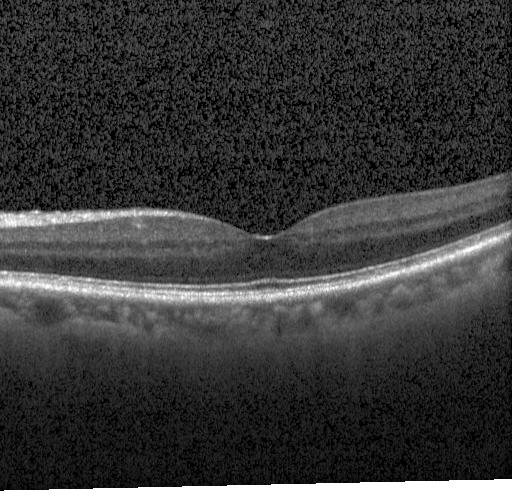 Acquired on a Heidelberg Spectralis; retinal OCT B-scan; fovea-centered; spectral-domain optical coherence tomography
Impression: no choroidal neovascularization, diabetic macular edema, or drusen.